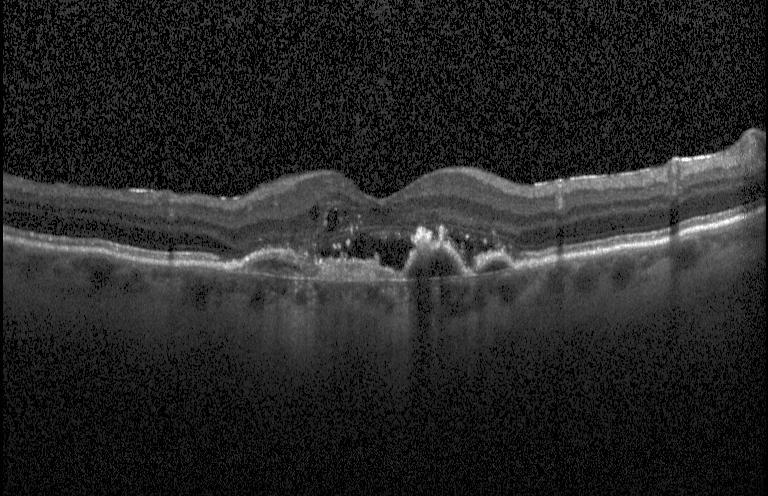
Spectral-domain OCT, optical coherence tomography scan, centered on the fovea, acquired on a Heidelberg Spectralis
A choroidal neovascular membrane.